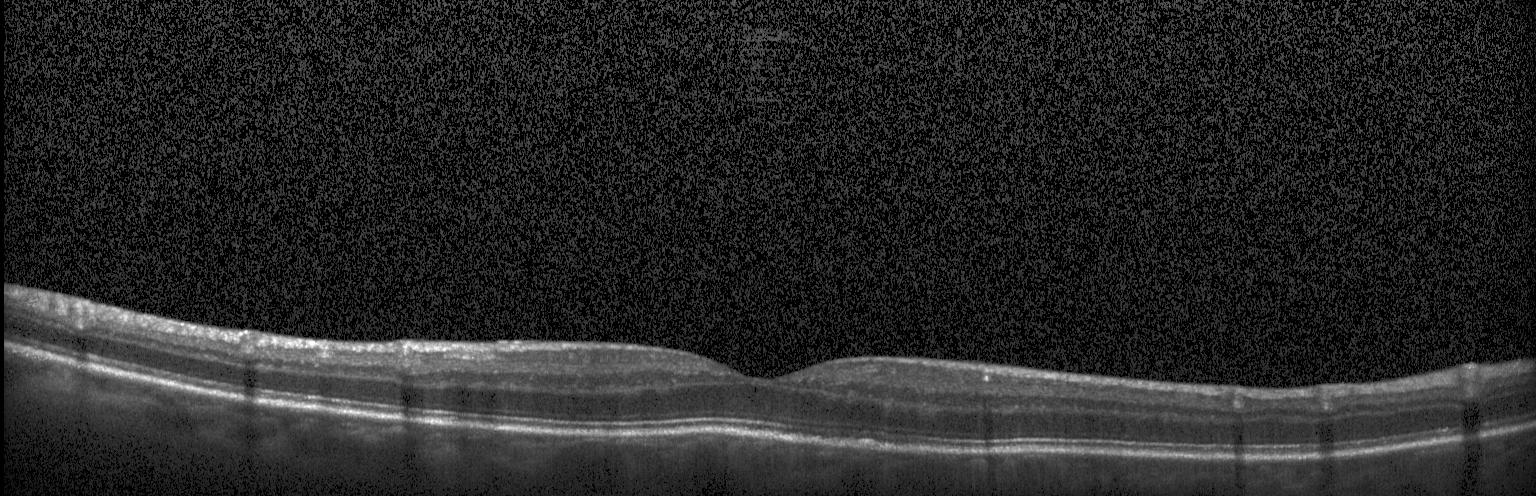
Heidelberg Spectralis · retinal OCT B-scan.
Dx: no choroidal neovascularization, diabetic macular edema, or drusen.